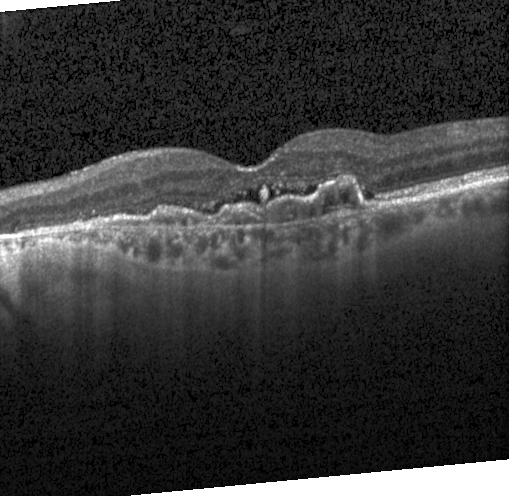
Spectral-domain OCT B-scan: choroidal neovascularization (CNV).